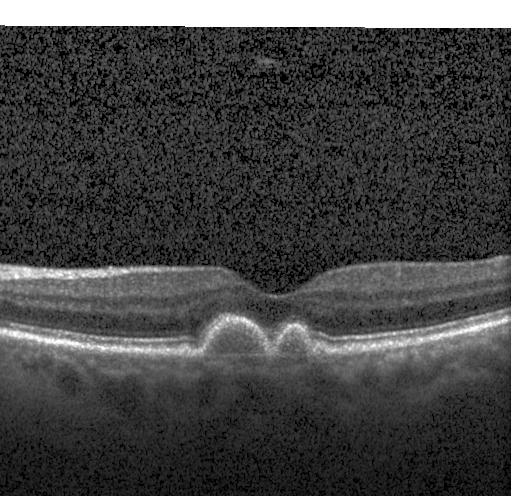 Instrument: Heidelberg Spectralis, optical coherence tomography B-scan. This B-scan demonstrates multiple drusen.